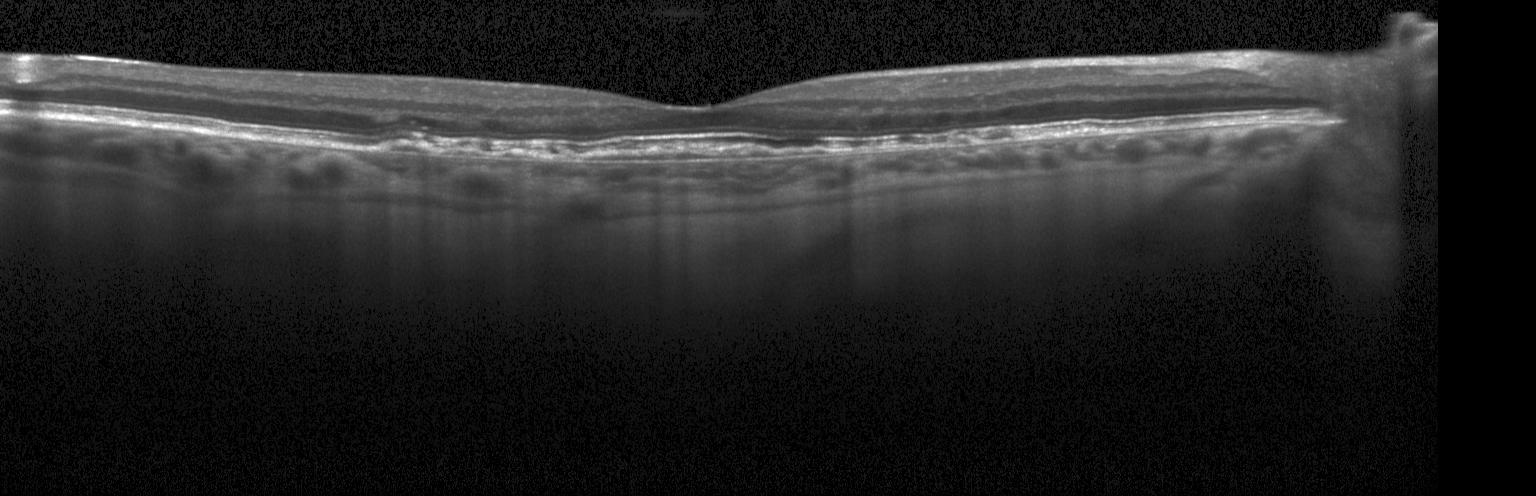 Impression: choroidal neovascularization.